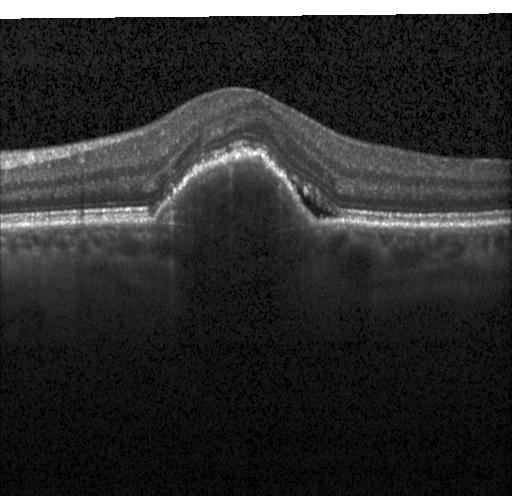
OCT line scan.
Diagnosis: a choroidal neovascular membrane.